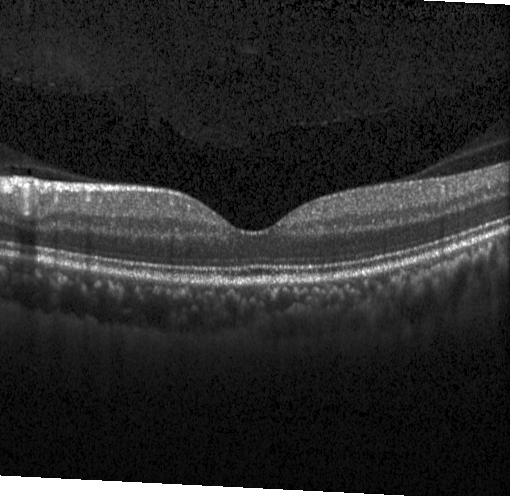
Macular scan · SD-OCT · acquired on a Heidelberg Spectralis · optical coherence tomography scan. This B-scan demonstrates no CNV, no DME, and no drusen.